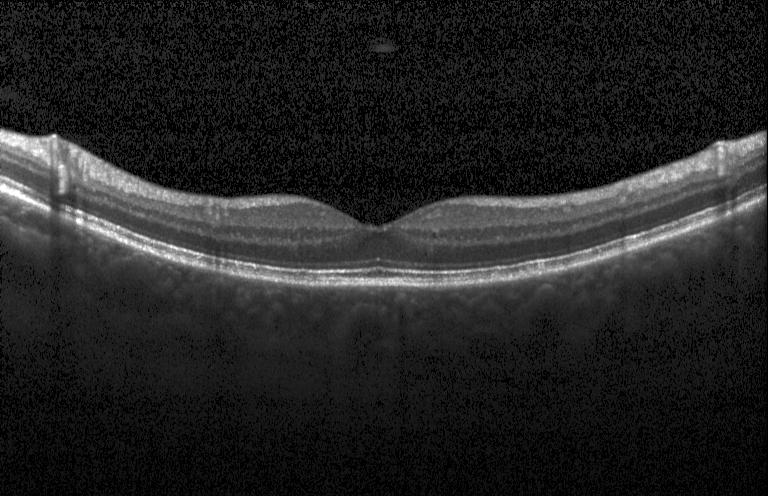

Macular scan · optical coherence tomography B-scan · SD-OCT.
Macular OCT: no choroidal neovascularization, diabetic macular edema, or drusen.